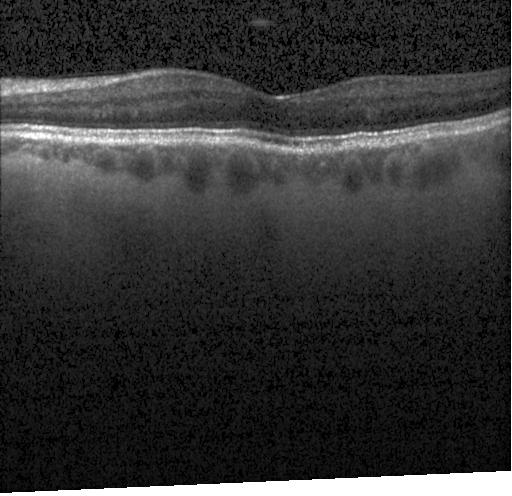
OCT finding: no choroidal neovascularization, diabetic macular edema, or drusen.